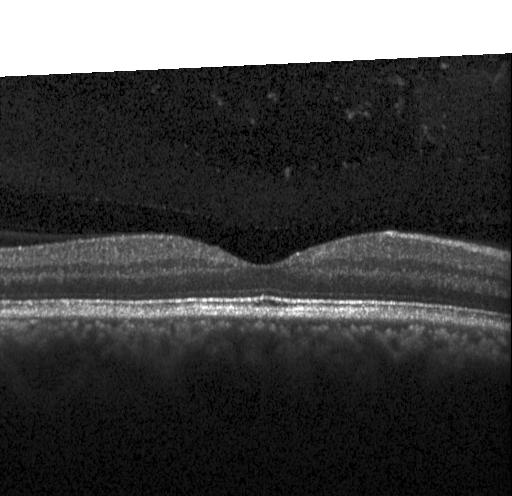 OCT finding: no evidence of CNV, DME, or drusen.